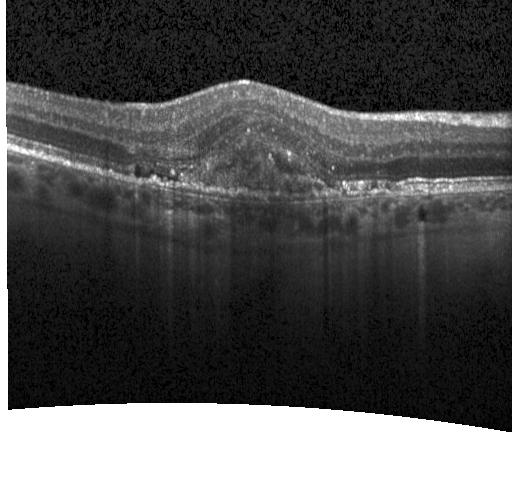

Finding: a choroidal neovascular membrane.